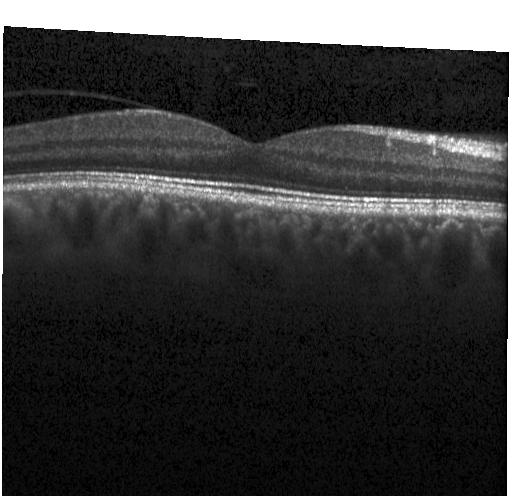

Spectral-domain OCT; Heidelberg Spectralis; optical coherence tomography scan — Macular OCT: neither choroidal neovascularization, diabetic macular edema, nor drusen.